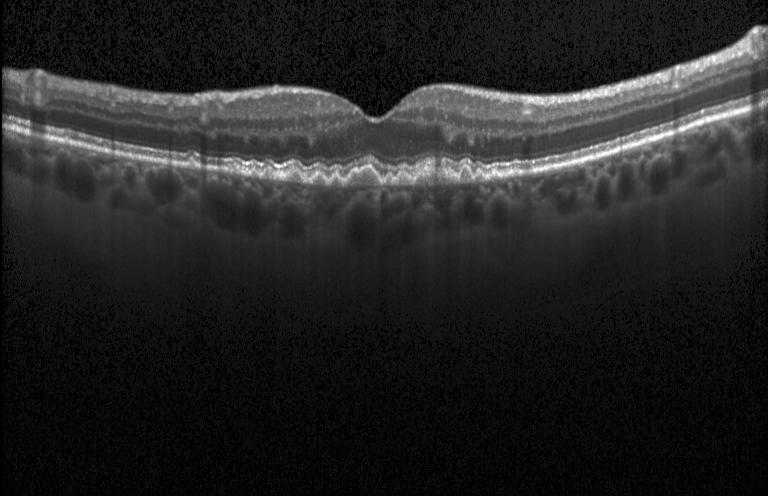
Drusen.